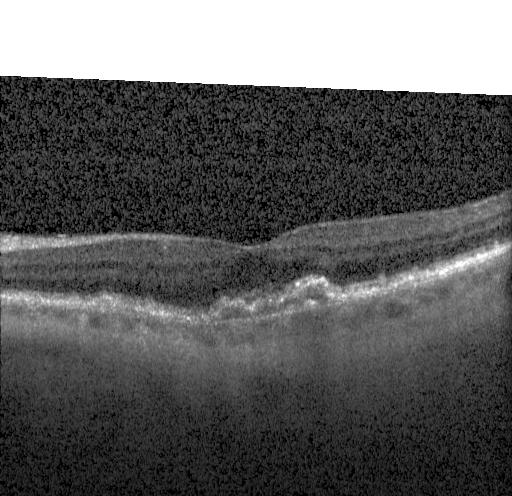

Macular OCT demonstrating a choroidal neovascular membrane.